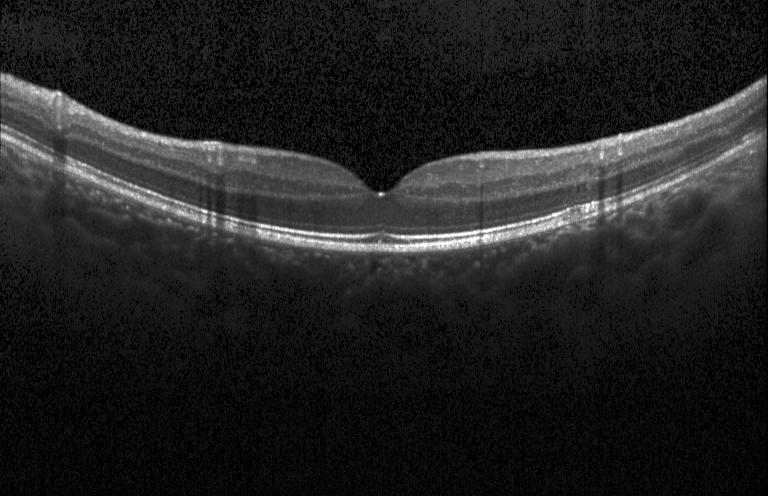
Retinal OCT cross-section.
Dx: no evidence of CNV, DME, or drusen.